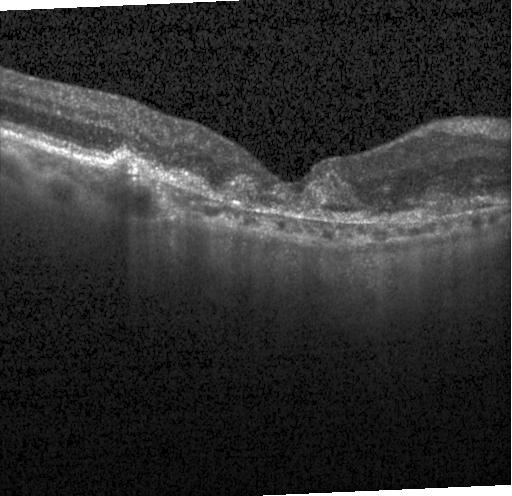
OCT line scan; through the macula; instrument: Heidelberg Spectralis.
The scan shows CNV.